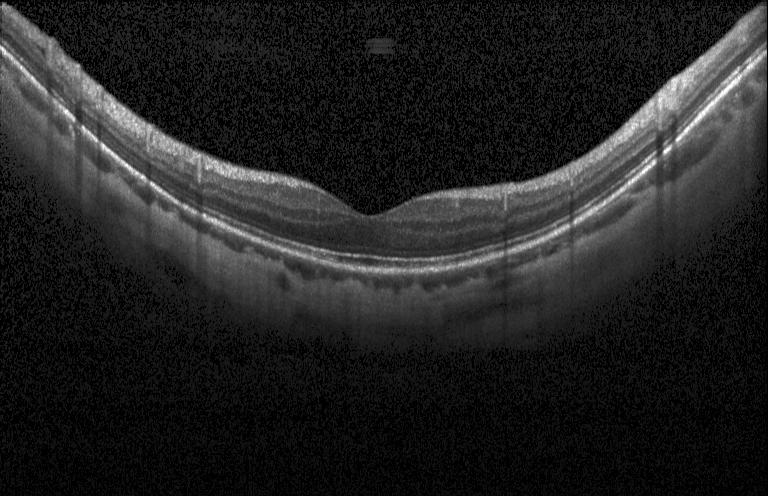

OCT line scan, SD-OCT
Assessment: neither CNV, DME, nor drusen.